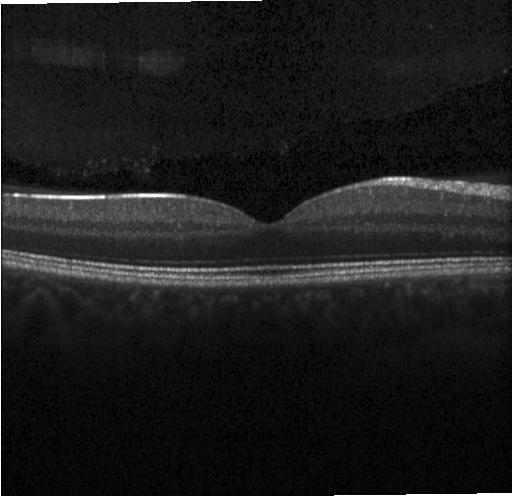

OCT scan showing no evidence of CNV, DME, or drusen.